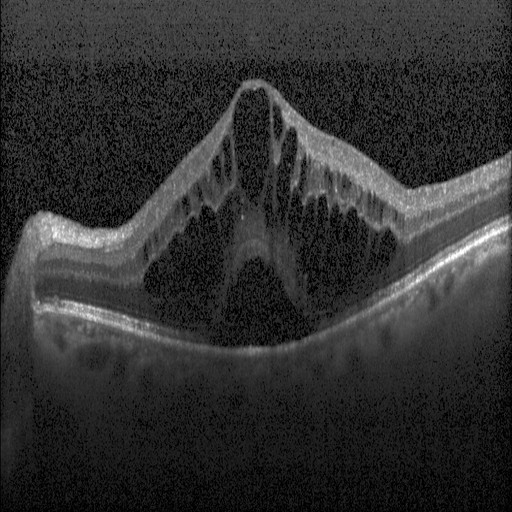
Through the macula. Spectral-domain optical coherence tomography. OCT line scan. Instrument: Heidelberg Spectralis — The scan shows DME.